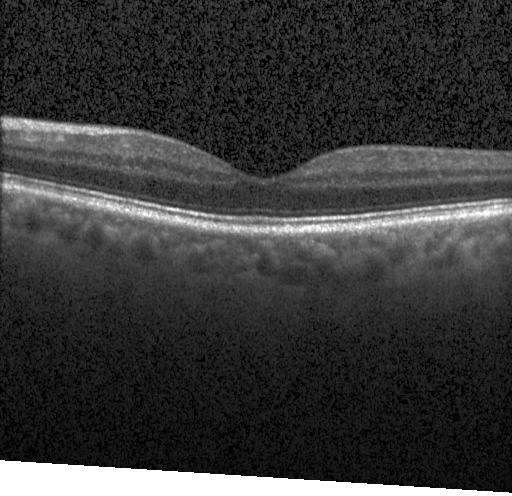 Dx: neither choroidal neovascularization, diabetic macular edema, nor drusen.